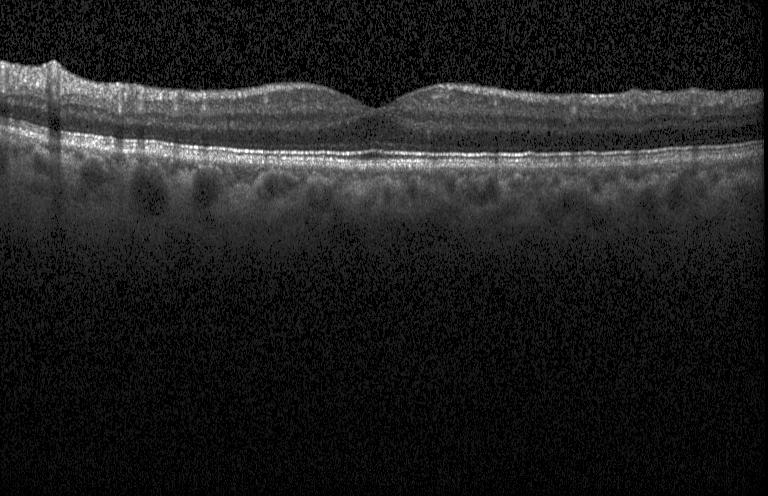 Retinal OCT cross-section showing no evidence of CNV, DME, or drusen.